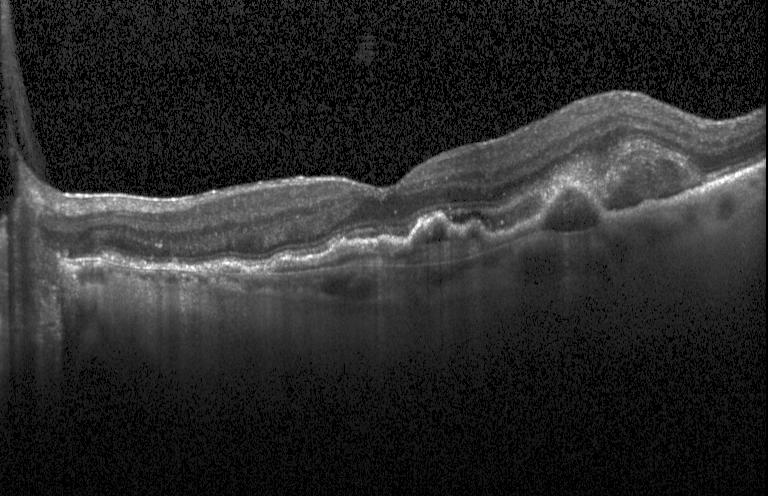 Spectral-domain OCT · through the macula · OCT B-scan · Heidelberg Spectralis. Diagnosis: choroidal neovascularization (CNV).